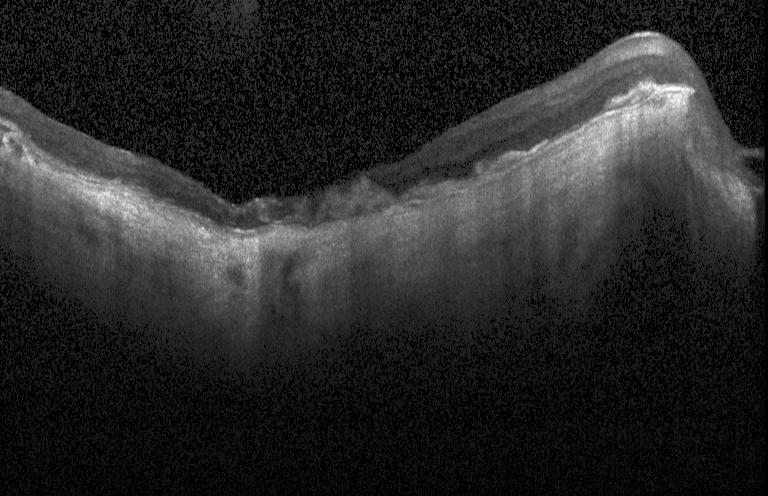 Heidelberg Spectralis · spectral-domain OCT · retinal OCT cross-section · macular scan
Macular OCT: a choroidal neovascular membrane.